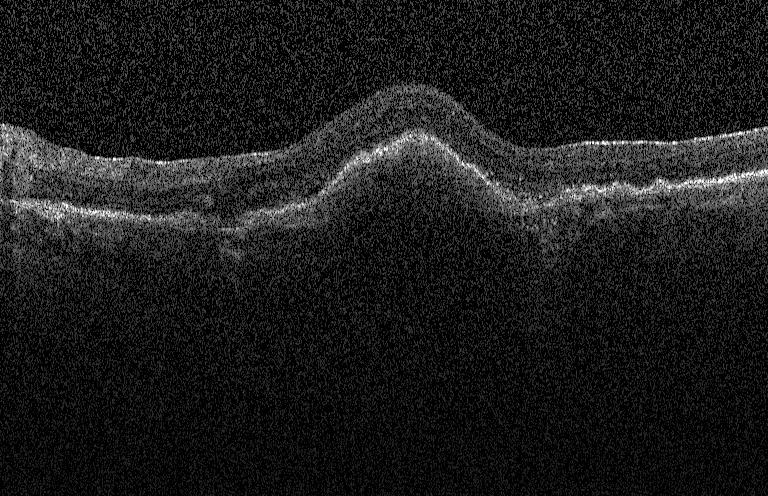

Heidelberg Spectralis. Fovea-centered. Retinal OCT cross-section — Impression: a choroidal neovascular membrane.